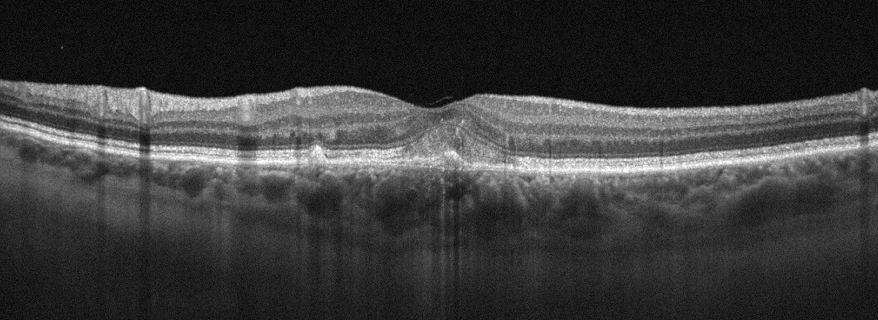

OCT scan showing age-related macular degeneration (AMD).